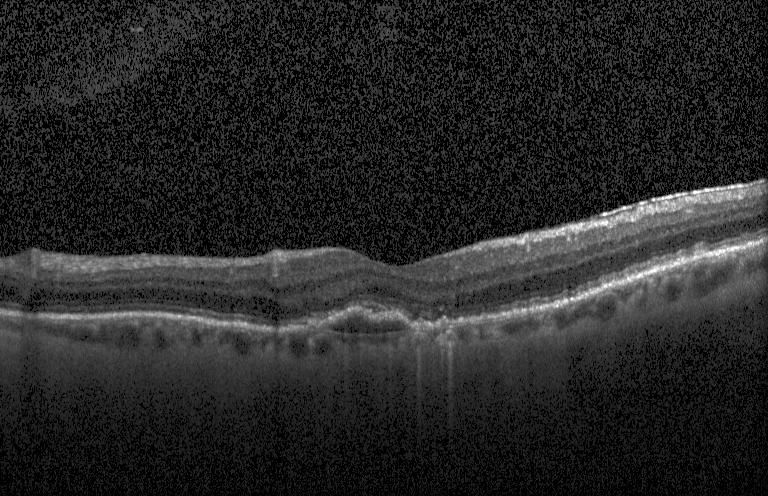 OCT line scan
Impression: choroidal neovascularization (CNV).